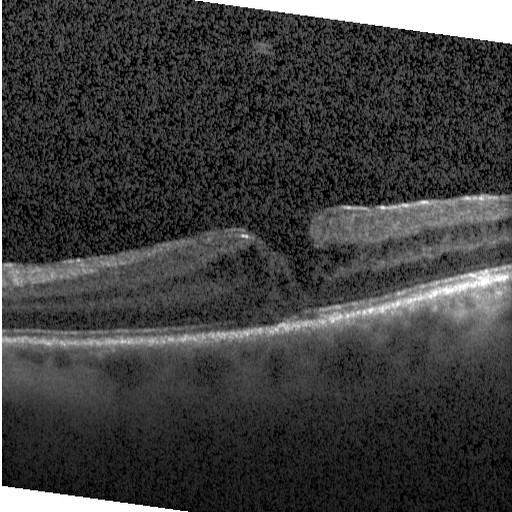
Spectral-domain OCT B-scan: diabetic macular edema.